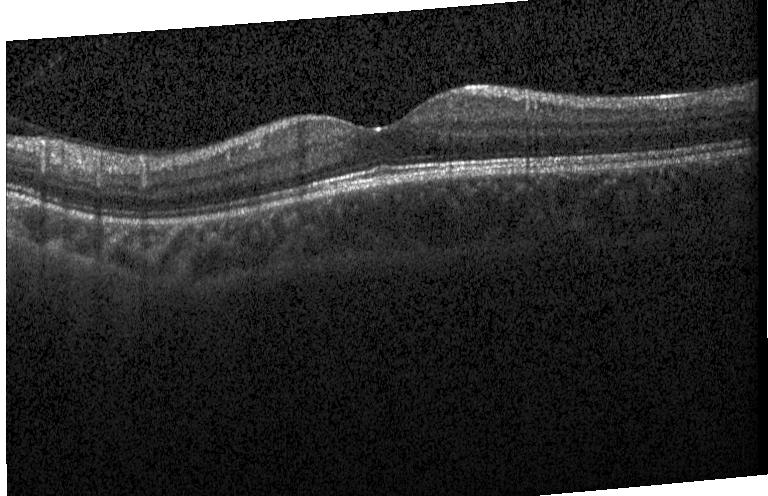

OCT line scan. Finding: no CNV, no DME, and no drusen.